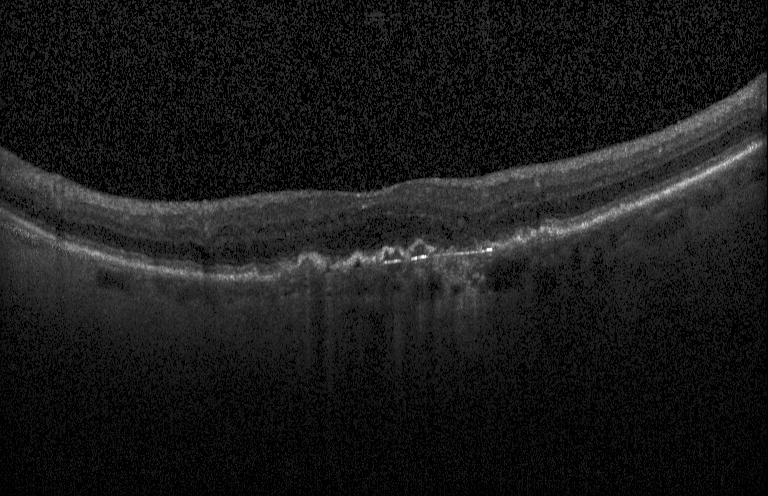 Heidelberg Spectralis · SD-OCT · centered on the fovea · optical coherence tomography scan. Diagnosis: a choroidal neovascular membrane.